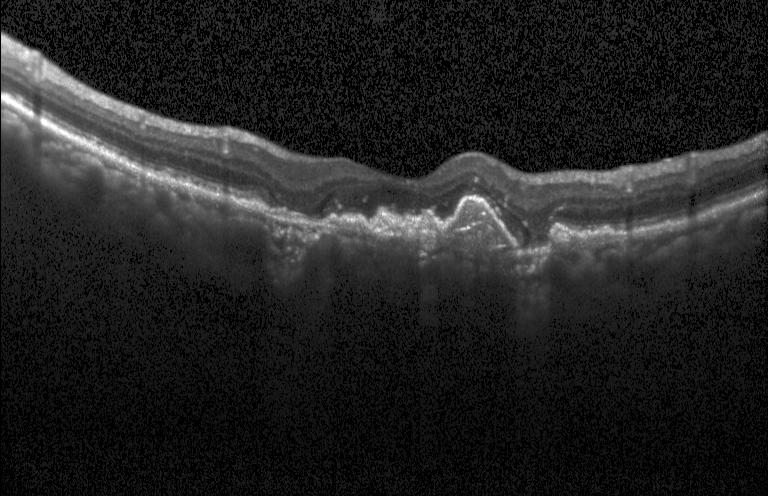
SD-OCT · instrument: Heidelberg Spectralis · optical coherence tomography scan · fovea-centered.
Impression: choroidal neovascularization (CNV).